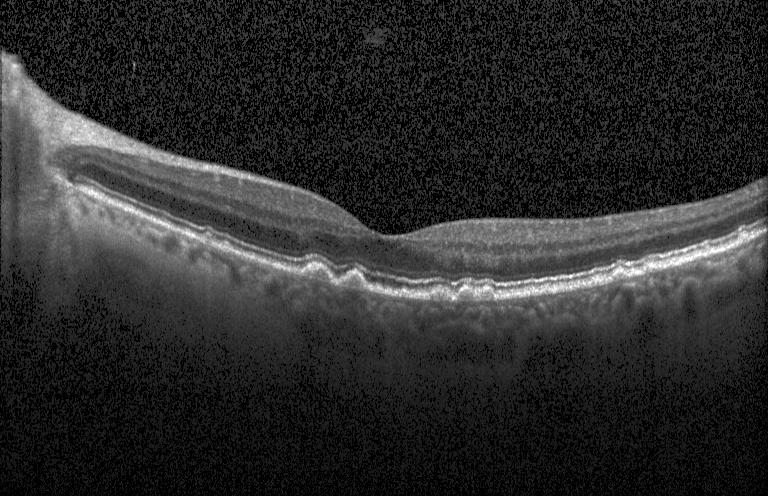

Fovea-centered. Retinal OCT cross-section — This B-scan demonstrates sub-RPE drusenoid deposits.